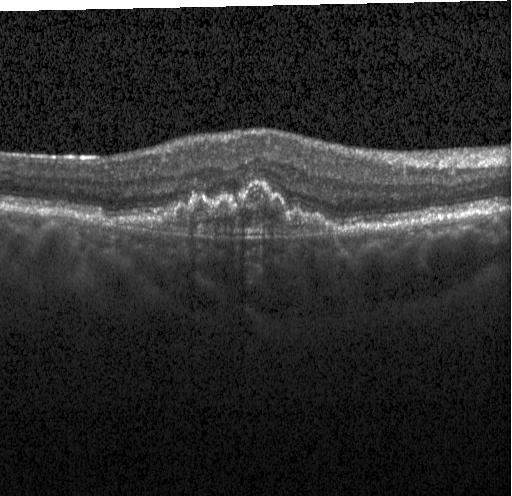

OCT finding: choroidal neovascularization (CNV).